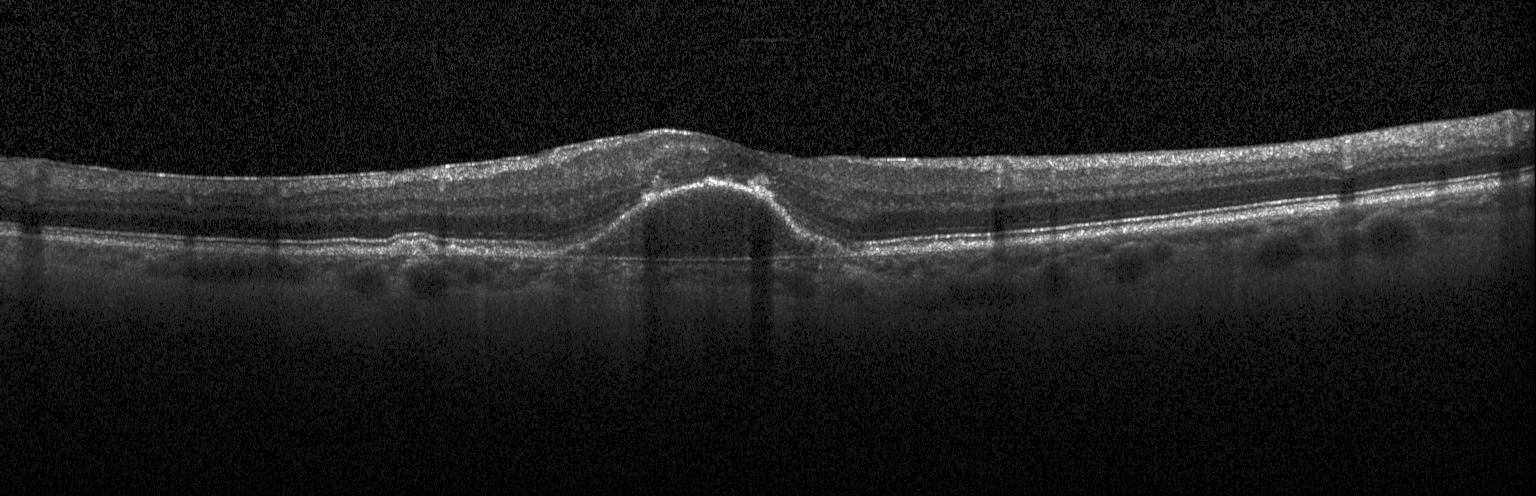
Centered on the fovea. Instrument: Heidelberg Spectralis. Optical coherence tomography scan.
This B-scan demonstrates choroidal neovascularization.